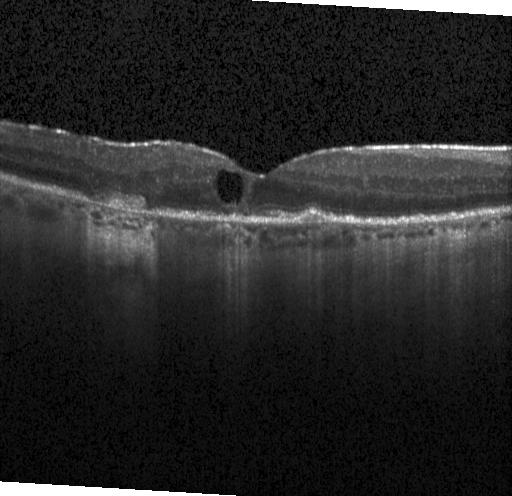
Heidelberg Spectralis OCT system · SD-OCT · optical coherence tomography B-scan — Impression: choroidal neovascularization.